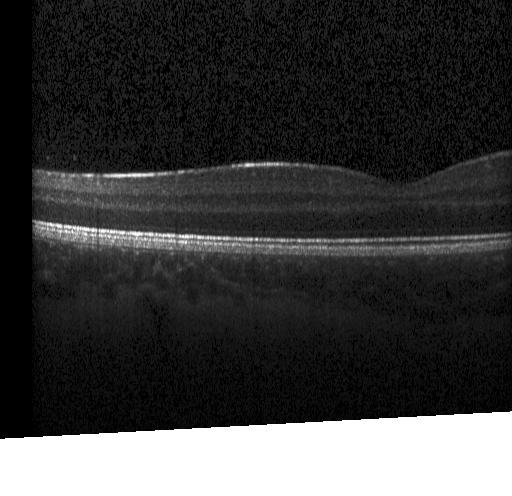 Finding: no CNV, no DME, and no drusen.